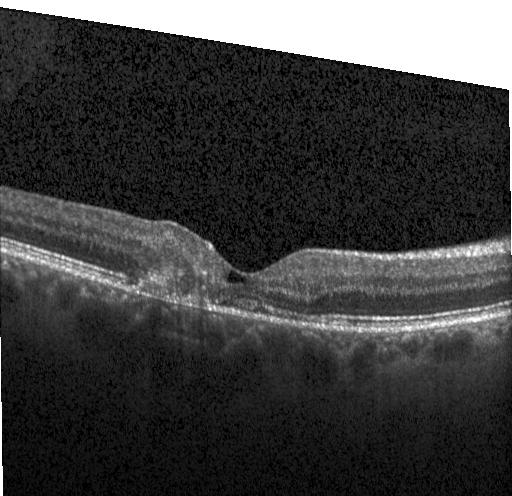
Diagnosis: choroidal neovascularization.